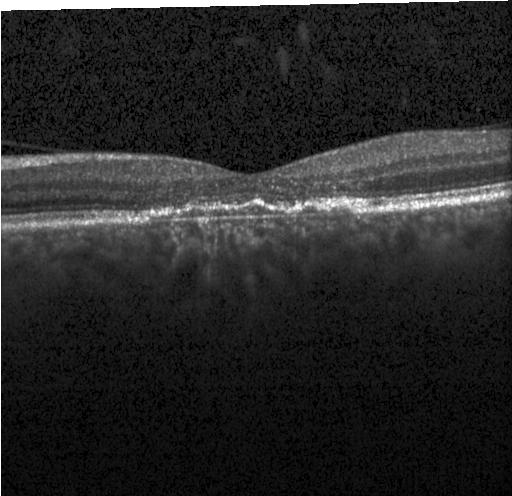 Heidelberg Spectralis, retinal OCT B-scan.
This B-scan demonstrates a choroidal neovascular membrane.